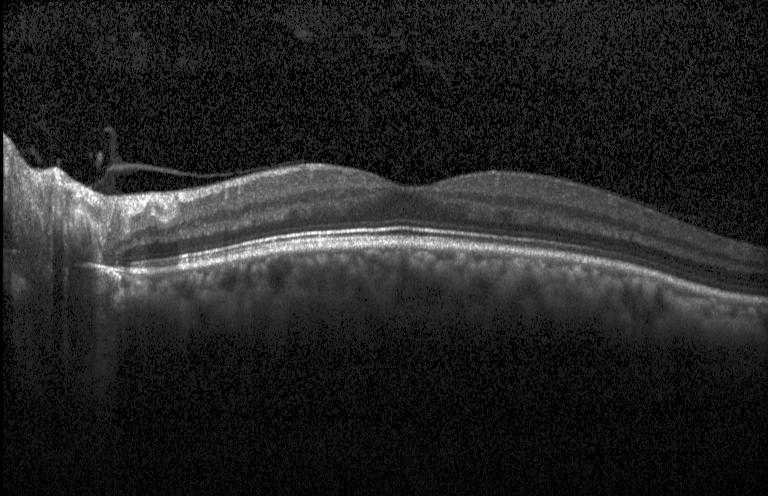 Optical coherence tomography scan; through the macula; spectral-domain optical coherence tomography; Heidelberg Spectralis OCT system
No evidence of choroidal neovascularization, diabetic macular edema, or drusen.